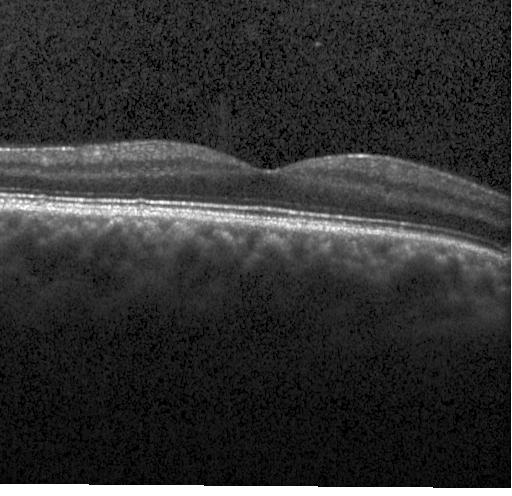

Dx: no evidence of choroidal neovascularization, diabetic macular edema, or drusen.